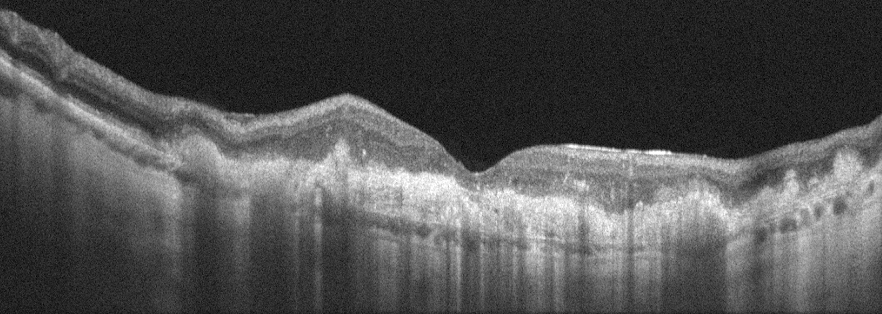

Oculus sinister. Retinal OCT cross-section — Finding: AMD.